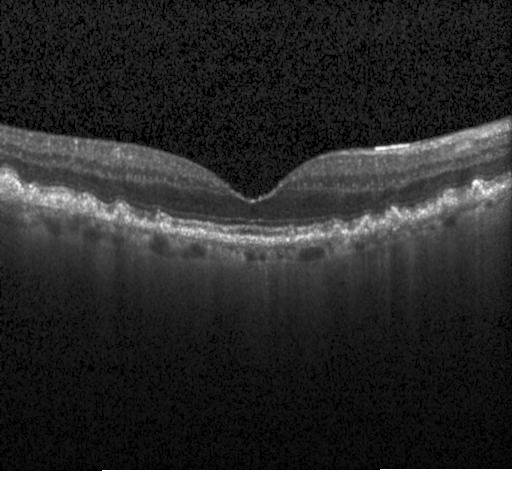
Macular OCT: drusen.